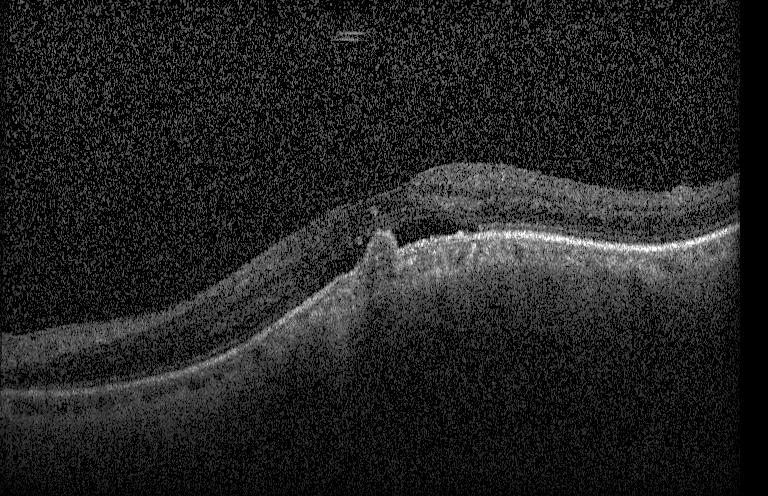

Instrument: Heidelberg Spectralis. SD-OCT. Retinal OCT B-scan
Impression: a choroidal neovascular membrane.